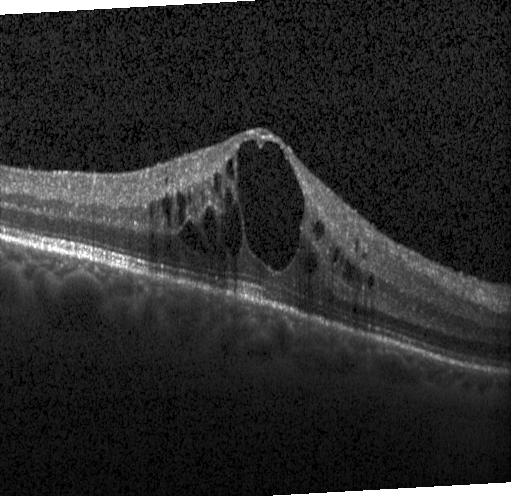 Impression: diabetic macular edema (DME).